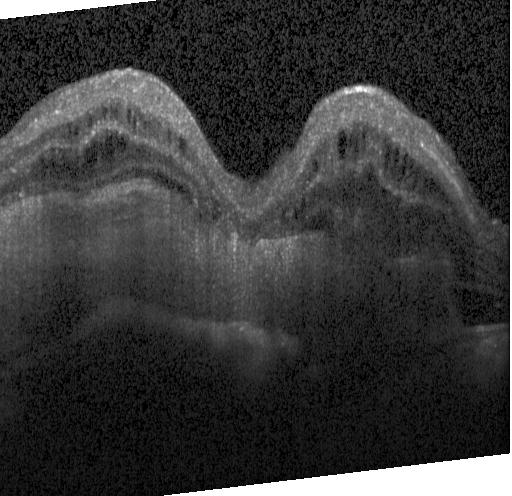

Macular scan · Heidelberg Spectralis OCT system · spectral-domain optical coherence tomography · retinal OCT B-scan
The scan shows a choroidal neovascular membrane.